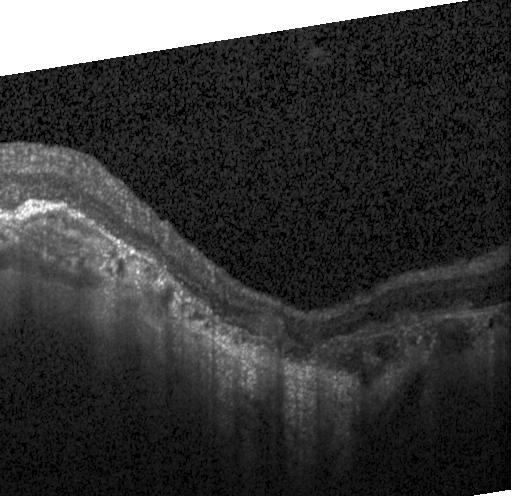 Acquired on a Heidelberg Spectralis. Horizontal scan through the fovea. Optical coherence tomography scan. Spectral-domain OCT
The scan shows a choroidal neovascular membrane.